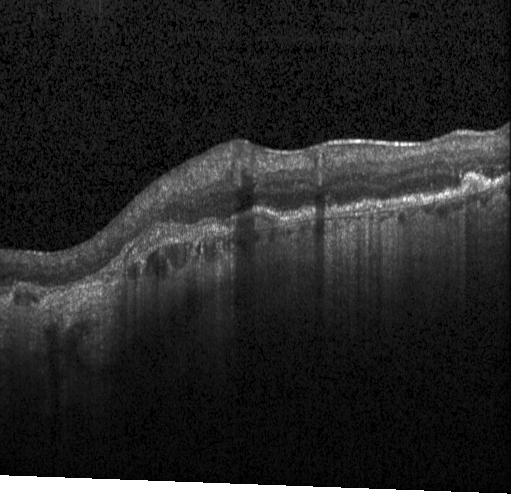
Impression: a choroidal neovascular membrane.